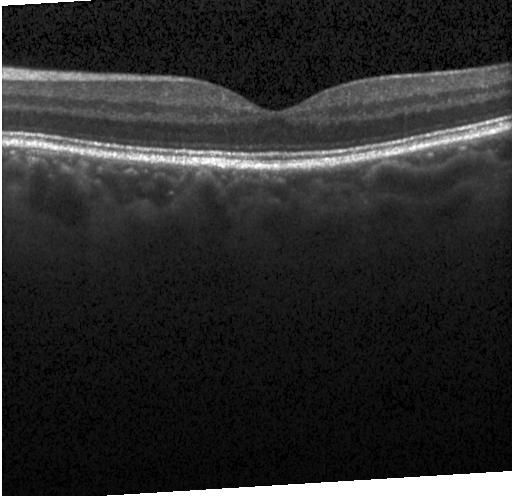
Dx: no evidence of CNV, DME, or drusen.